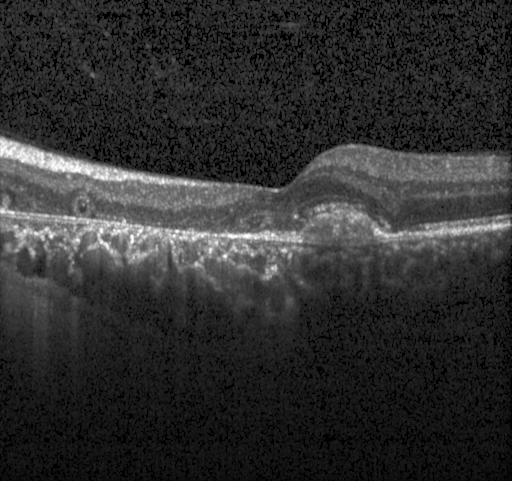

OCT line scan
Finding: CNV.